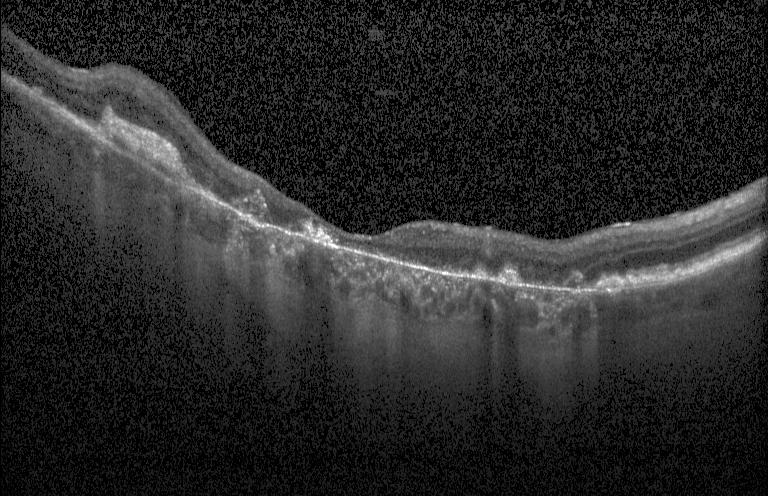 Optical coherence tomography scan
The scan shows choroidal neovascularization (CNV).